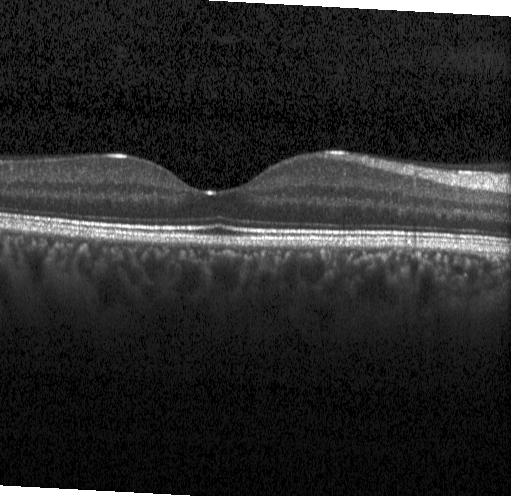
Impression: no choroidal neovascularization, no diabetic macular edema, and no drusen.